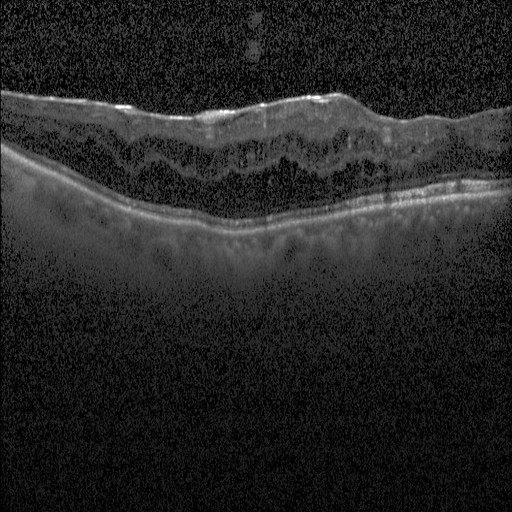
Spectral-domain optical coherence tomography · centered on the fovea · instrument: Heidelberg Spectralis · optical coherence tomography B-scan.
Assessment: diabetic macular edema (DME).